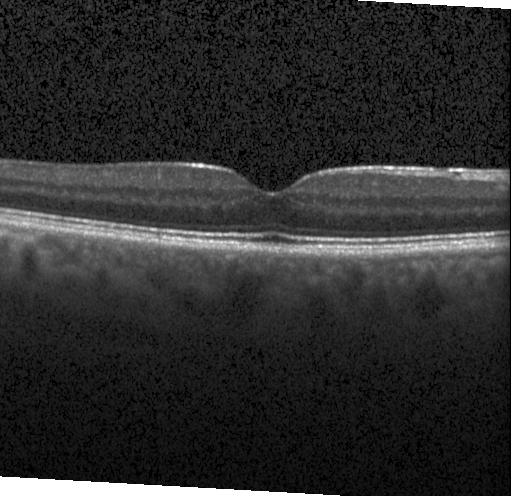 SD-OCT · optical coherence tomography B-scan. Impression: no CNV, no DME, and no drusen.